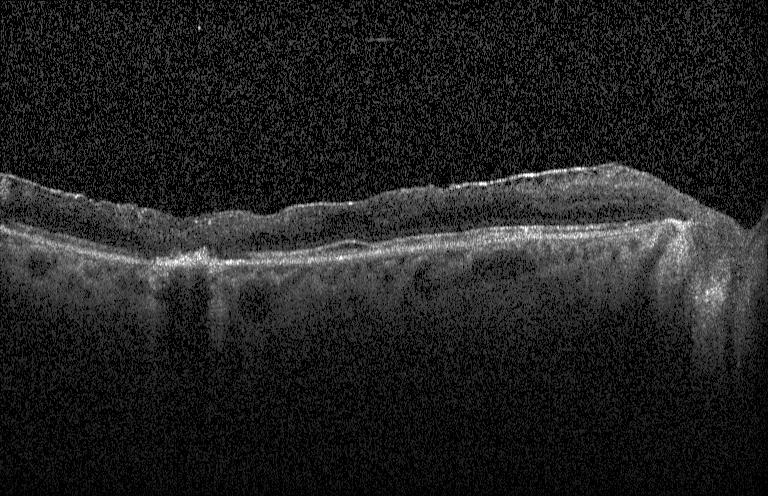 Macular OCT: CNV.